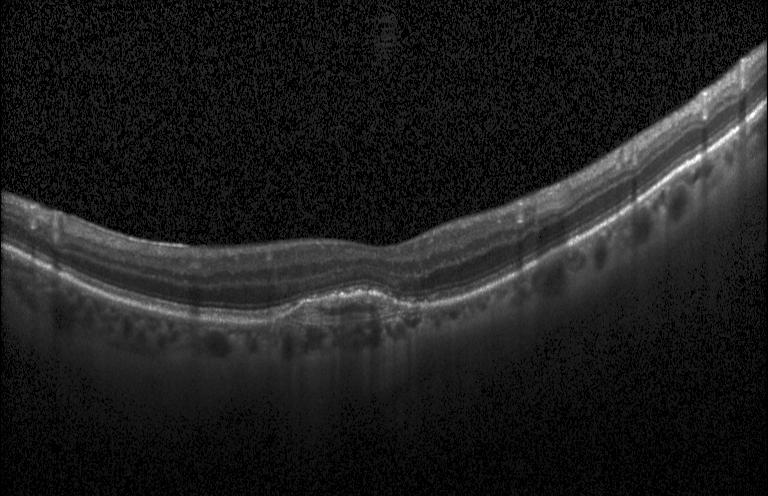 Retinal OCT cross-section showing a choroidal neovascular membrane.